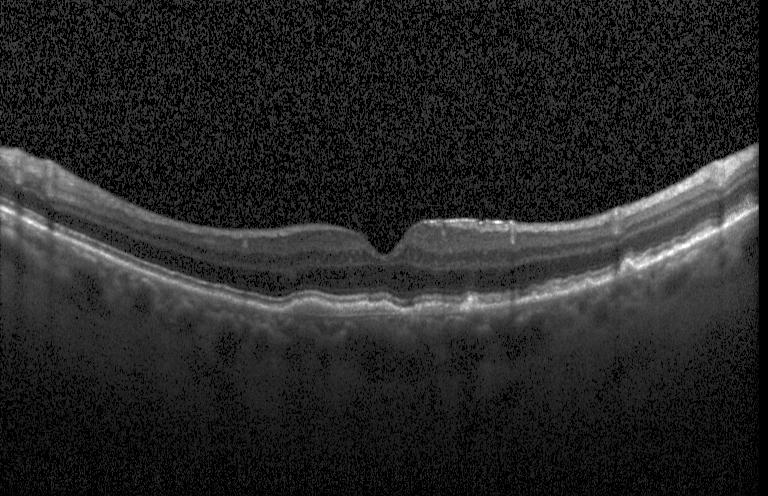

Acquired on a Heidelberg Spectralis; optical coherence tomography scan; fovea-centered; spectral-domain optical coherence tomography
Dx: choroidal neovascularization.